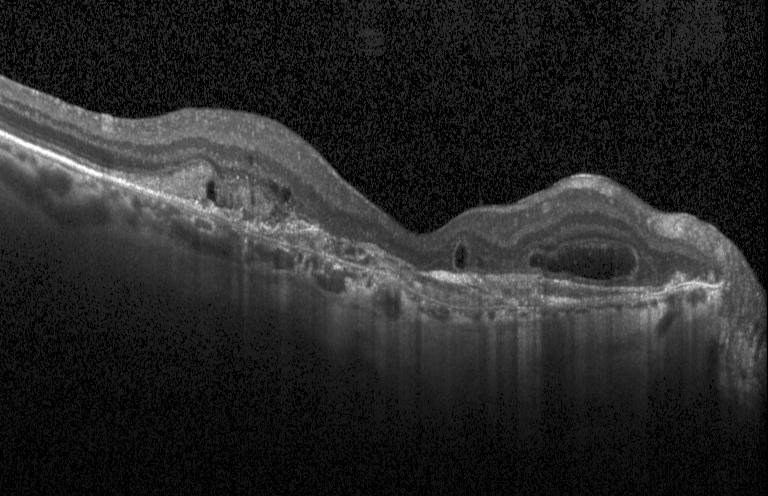
Dx: choroidal neovascularization.